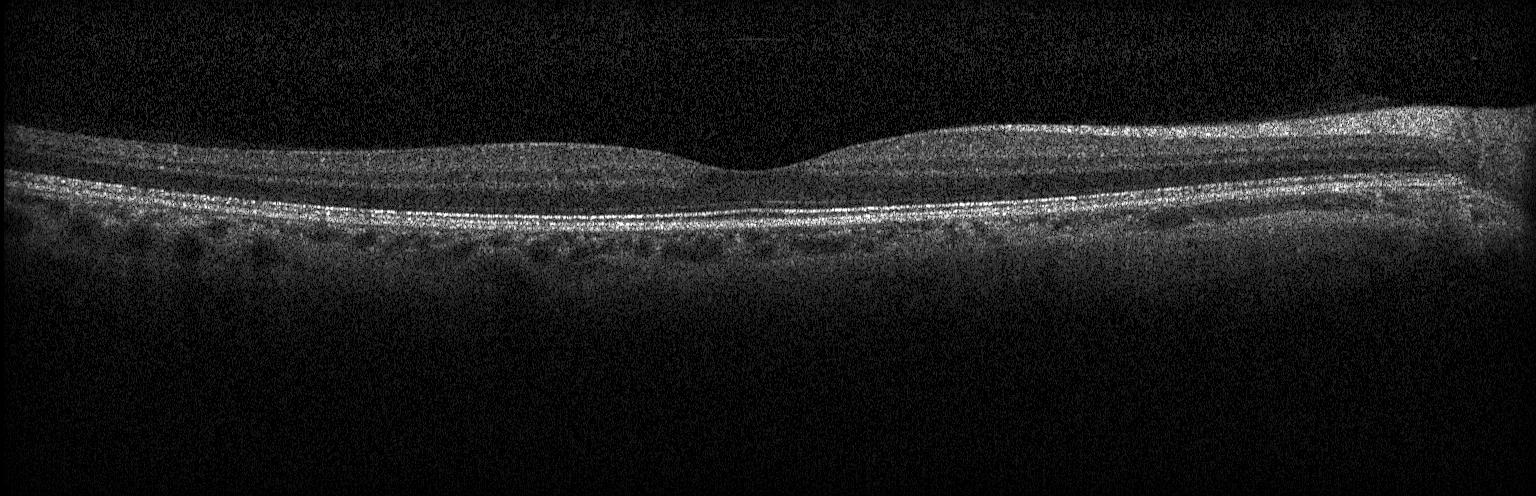

Macular OCT demonstrating no choroidal neovascularization, diabetic macular edema, or drusen.